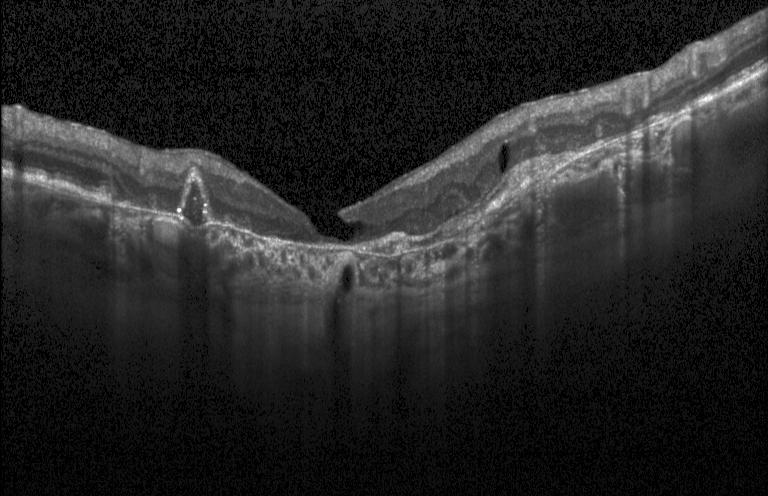
Instrument: Heidelberg Spectralis · SD-OCT · optical coherence tomography scan
The scan shows CNV.